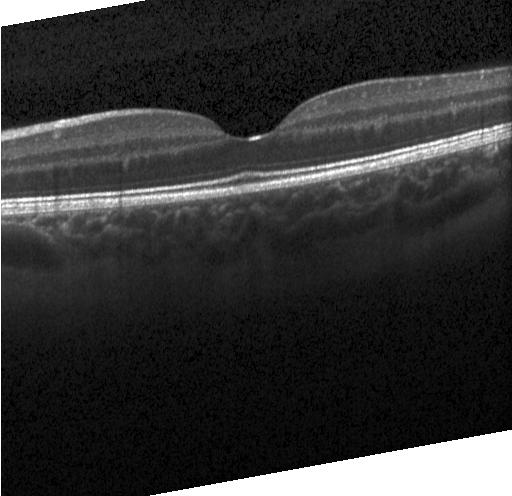

OCT B-scan — This B-scan demonstrates no choroidal neovascularization, no diabetic macular edema, and no drusen.